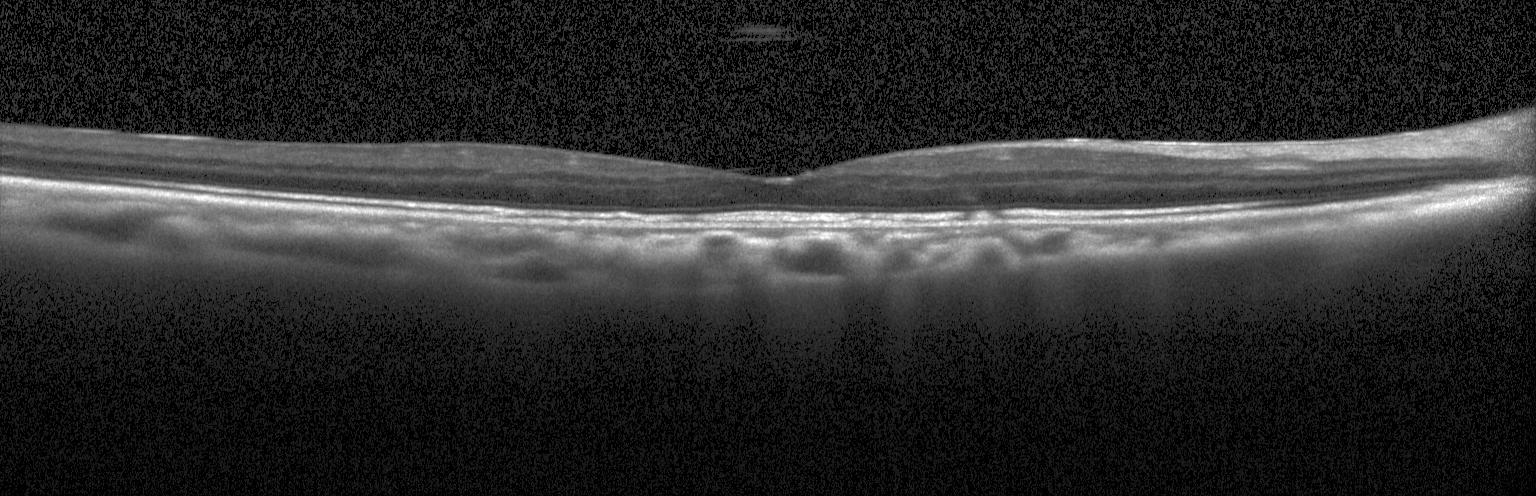 Dx: no choroidal neovascularization, diabetic macular edema, or drusen.